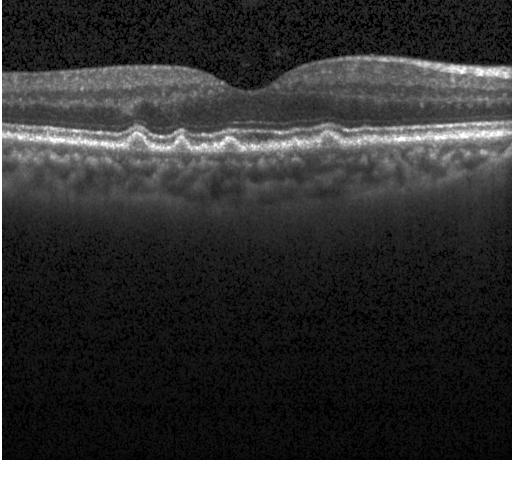
Assessment: drusen.